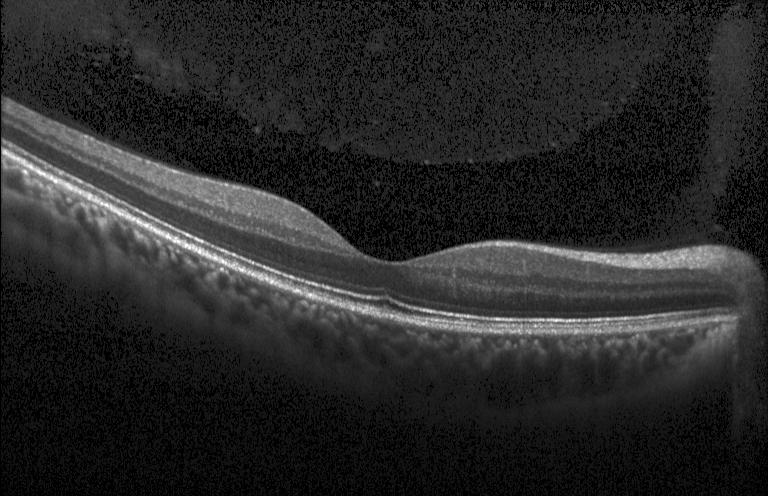
Retinal OCT cross-section · macular scan · Heidelberg Spectralis OCT system · spectral-domain OCT
Impression: no choroidal neovascularization, no diabetic macular edema, and no drusen.